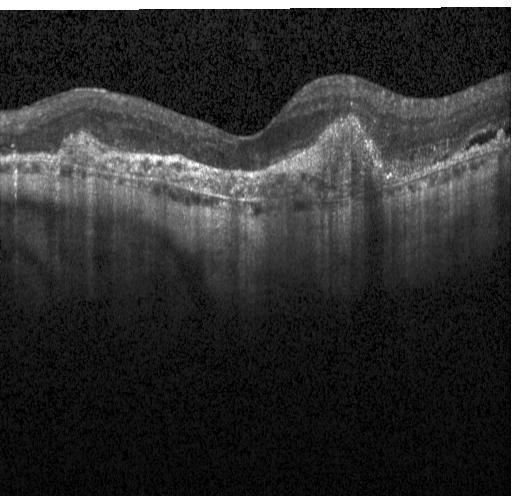
Retinal OCT B-scan · fovea-centered · Heidelberg Spectralis OCT system · spectral-domain OCT — Diagnosis: a choroidal neovascular membrane.